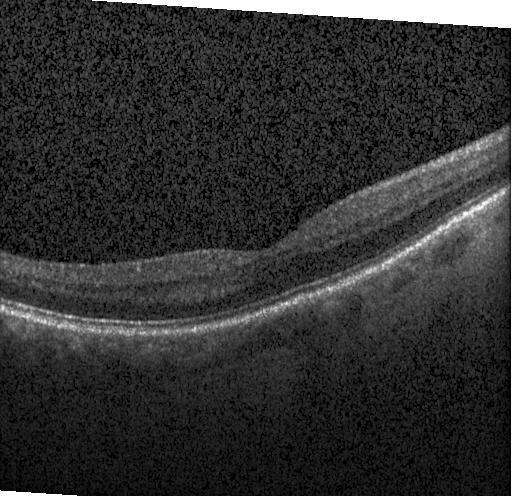 Optical coherence tomography scan; spectral-domain optical coherence tomography; instrument: Heidelberg Spectralis — Impression: no evidence of choroidal neovascularization, diabetic macular edema, or drusen.